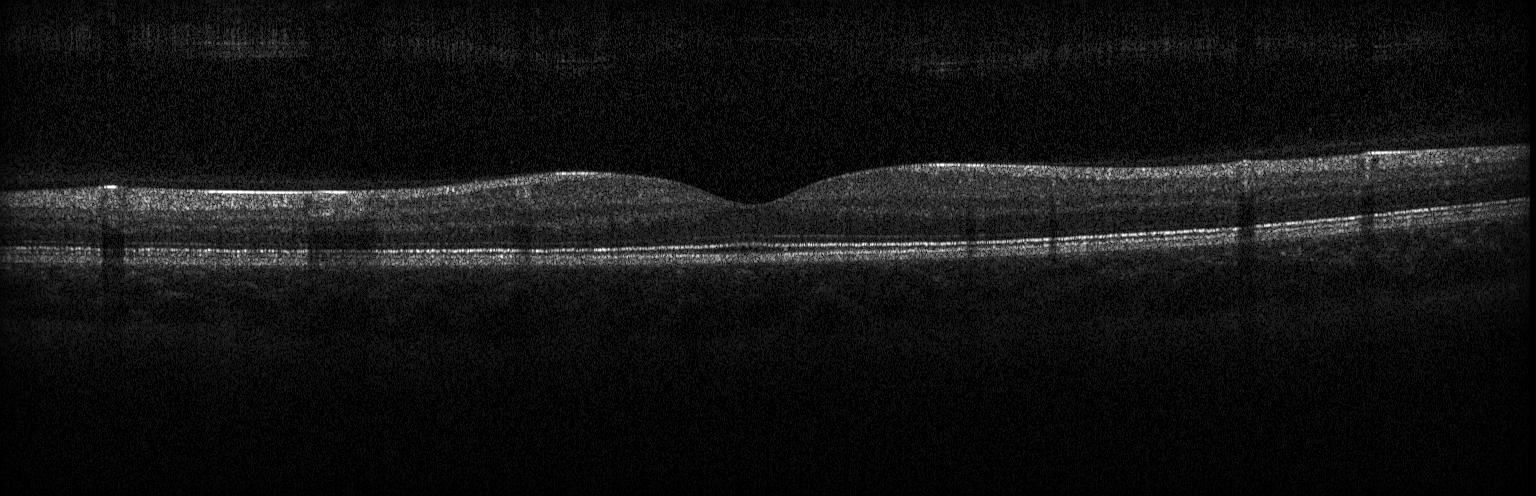
Instrument: Heidelberg Spectralis. Through the macula. Optical coherence tomography B-scan. Spectral-domain OCT.
This B-scan demonstrates no CNV, no DME, and no drusen.